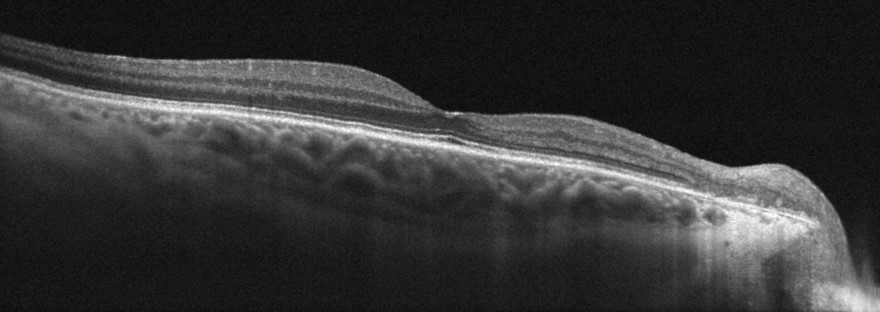 Retinal OCT cross-section.
Impression: no AMD, DME, ERM, RAO, RVO, or VID.